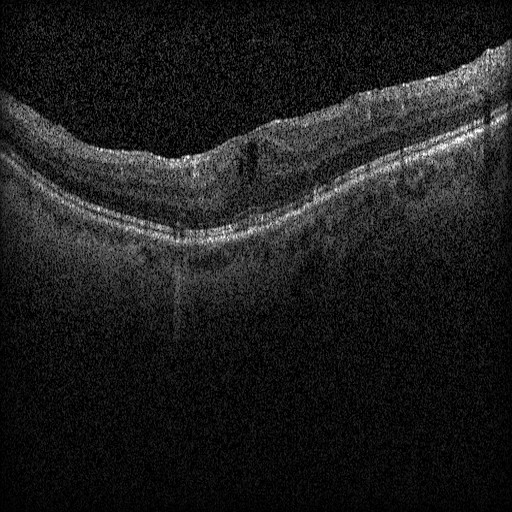 Retinal OCT B-scan; centered on the fovea
Diagnosis: DME.